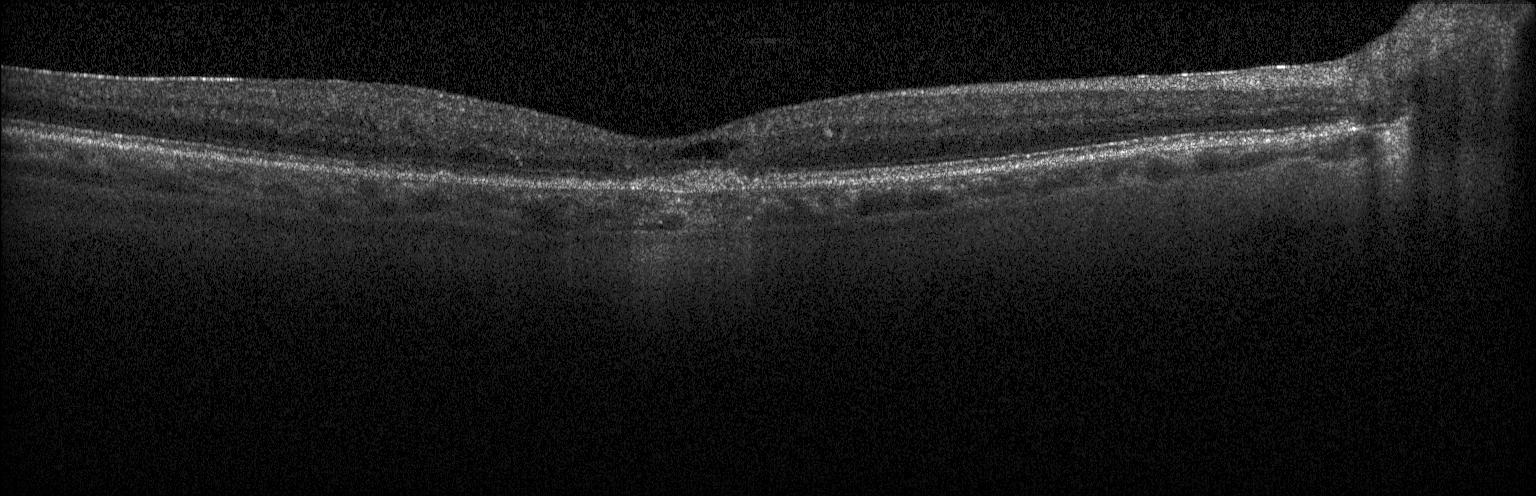
Acquired on a Heidelberg Spectralis, macular scan, spectral-domain optical coherence tomography, retinal OCT cross-section.
Impression: a choroidal neovascular membrane.